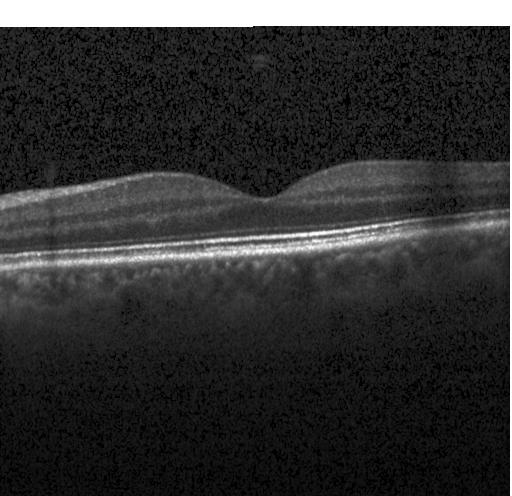
Retinal OCT B-scan, macular scan — Impression: no evidence of choroidal neovascularization, diabetic macular edema, or drusen.